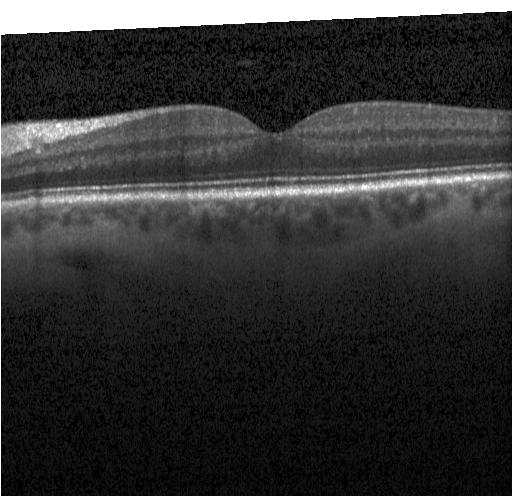 Optical coherence tomography scan · horizontal scan through the fovea
Impression: neither CNV, DME, nor drusen.